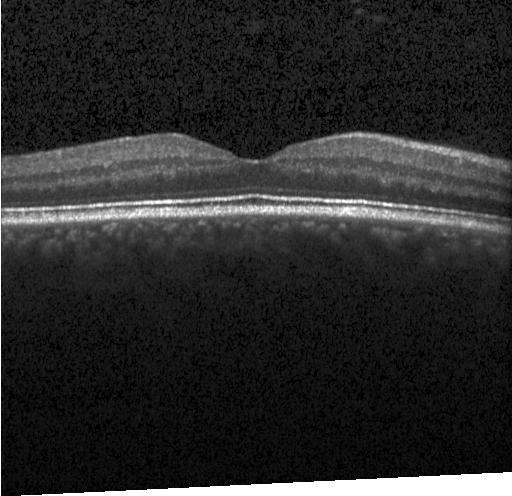
OCT B-scan · fovea-centered
This B-scan demonstrates no CNV, DME, or drusen.